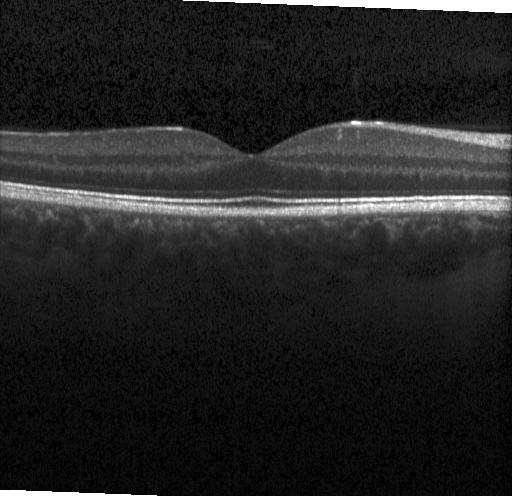 Retinal OCT cross-section; acquired on a Heidelberg Spectralis; spectral-domain OCT
The scan shows no choroidal neovascularization, diabetic macular edema, or drusen.